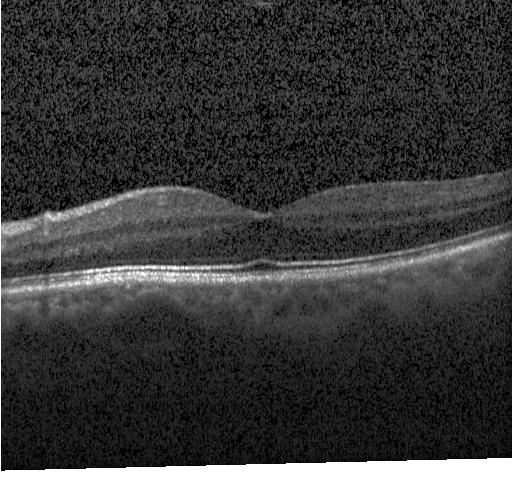 Centered on the fovea · acquired on a Heidelberg Spectralis · optical coherence tomography B-scan · SD-OCT — Impression: no choroidal neovascularization, no diabetic macular edema, and no drusen.